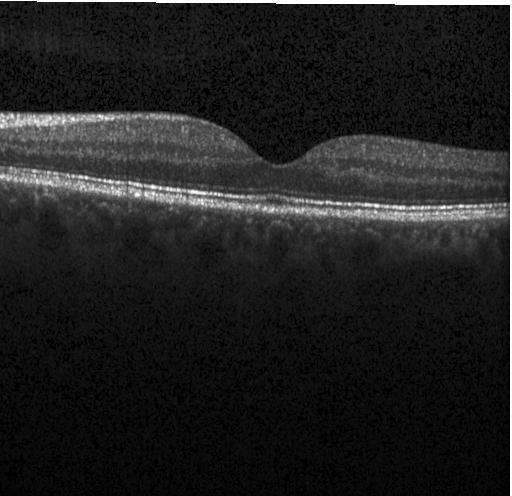

Through the macula, retinal OCT cross-section, spectral-domain optical coherence tomography. Finding: neither choroidal neovascularization, diabetic macular edema, nor drusen.